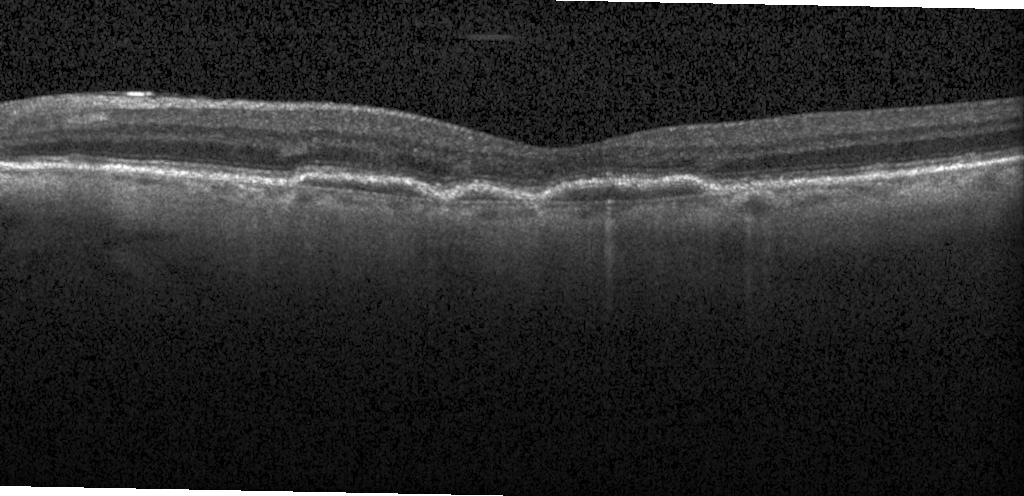

OCT finding: choroidal neovascularization.